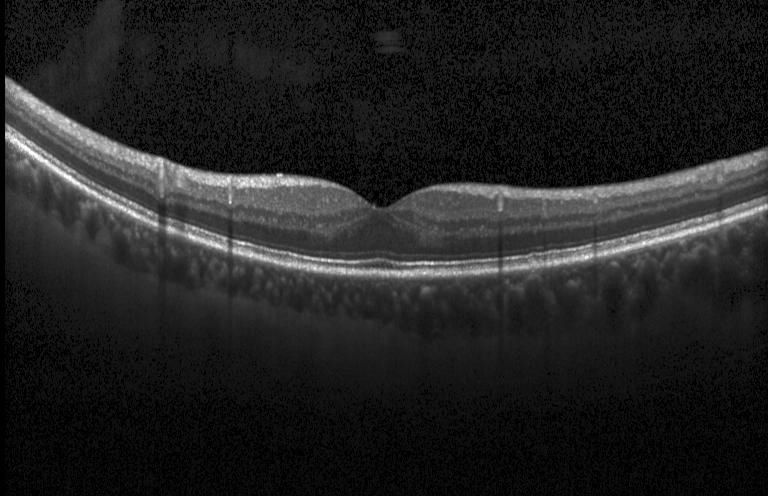 Heidelberg Spectralis OCT system, spectral-domain OCT, OCT line scan, through the macula. The scan shows neither CNV, DME, nor drusen.